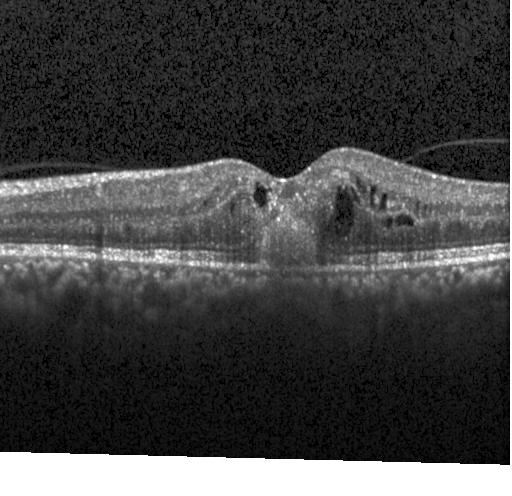

Optical coherence tomography B-scan · horizontal scan through the fovea · spectral-domain OCT — This B-scan demonstrates a choroidal neovascular membrane.